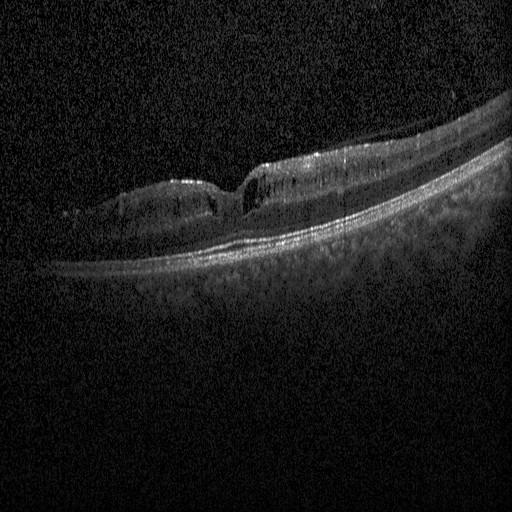 Optical coherence tomography B-scan — Finding: DME.